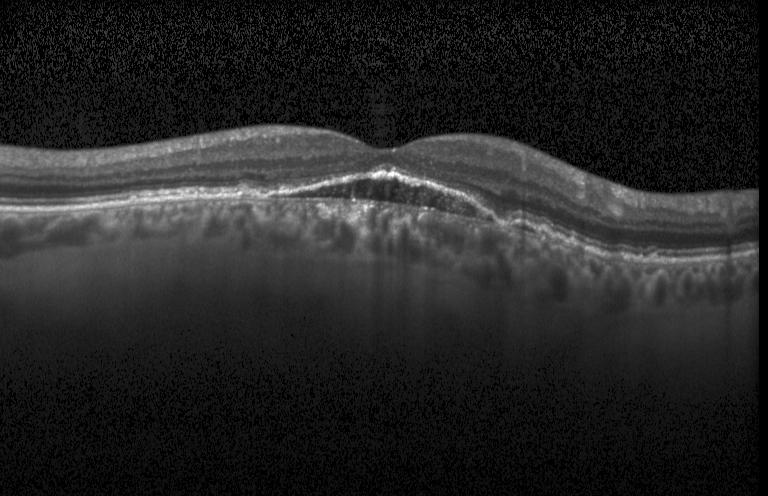
This B-scan demonstrates CNV.